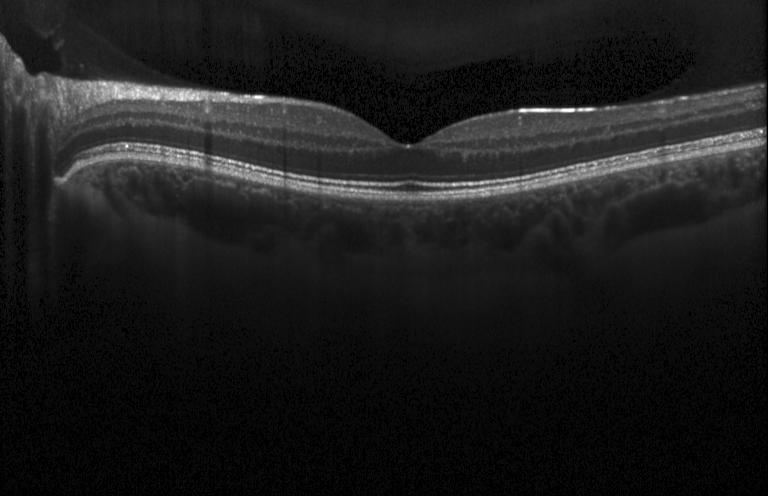

Dx: no CNV, DME, or drusen.